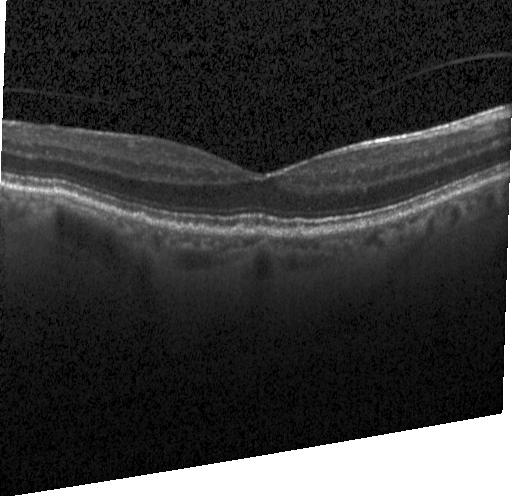 Spectral-domain OCT B-scan: sub-RPE drusenoid deposits.